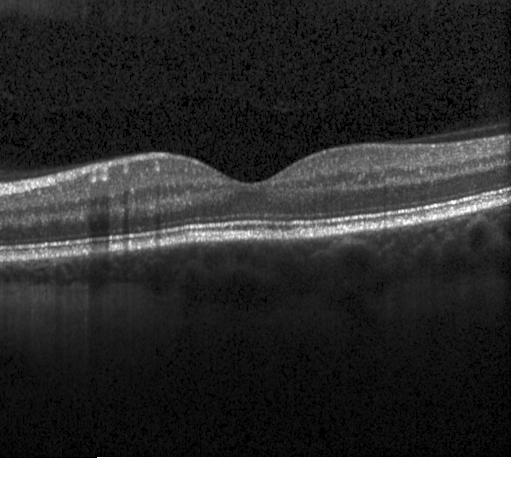 Retinal OCT cross-section showing no CNV, no DME, and no drusen.